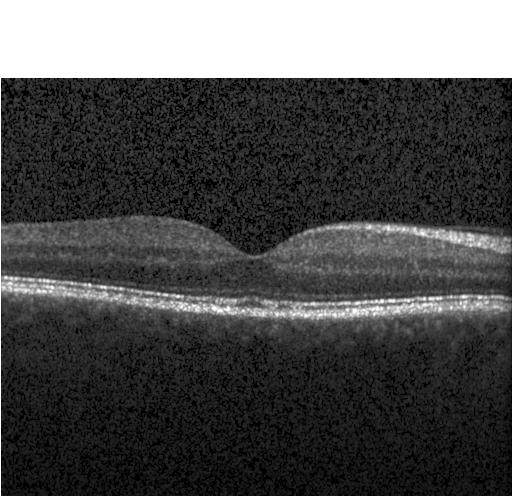 No CNV, DME, or drusen.